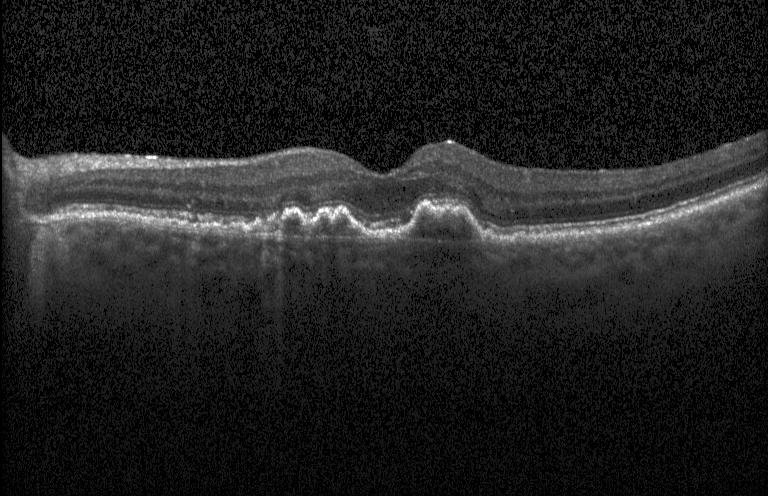

OCT line scan
Macular OCT: a choroidal neovascular membrane.